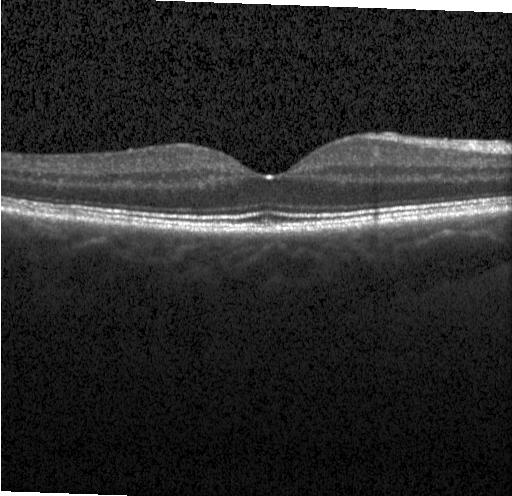 Retinal OCT B-scan.
Impression: no evidence of choroidal neovascularization, diabetic macular edema, or drusen.